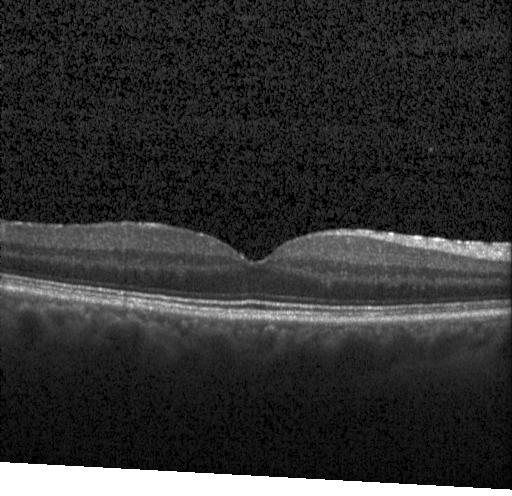 Dx: no choroidal neovascularization, no diabetic macular edema, and no drusen.